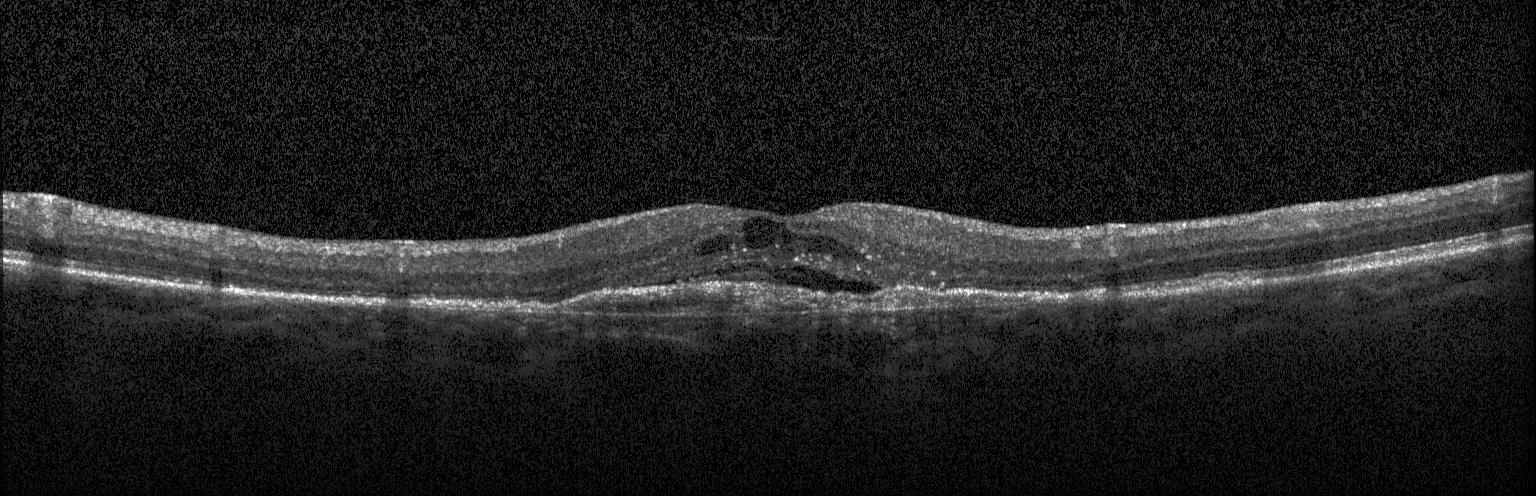
Optical coherence tomography B-scan
Assessment: a choroidal neovascular membrane.